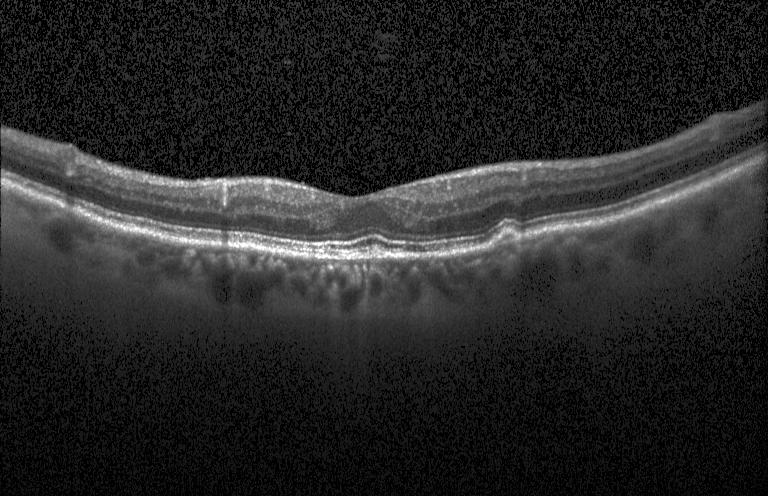 Finding: sub-RPE drusenoid deposits.